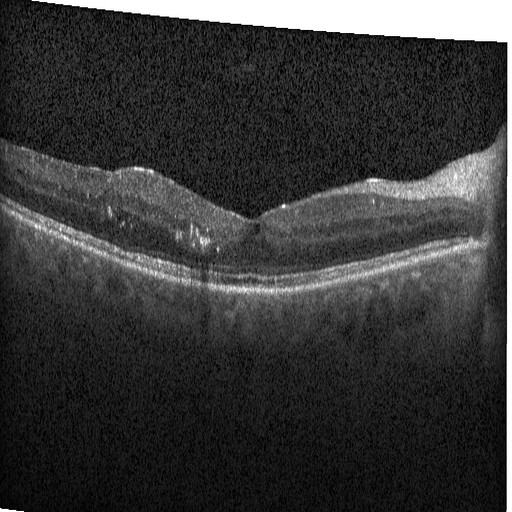

OCT line scan; Heidelberg Spectralis. The scan shows diabetic macular edema (DME).